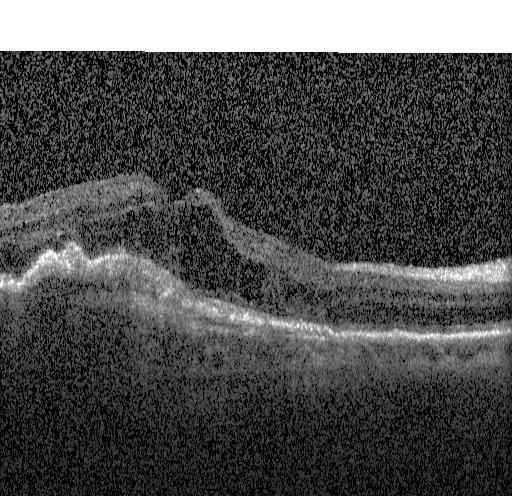 Acquired on a Heidelberg Spectralis, spectral-domain optical coherence tomography, retinal OCT cross-section.
Finding: a choroidal neovascular membrane.